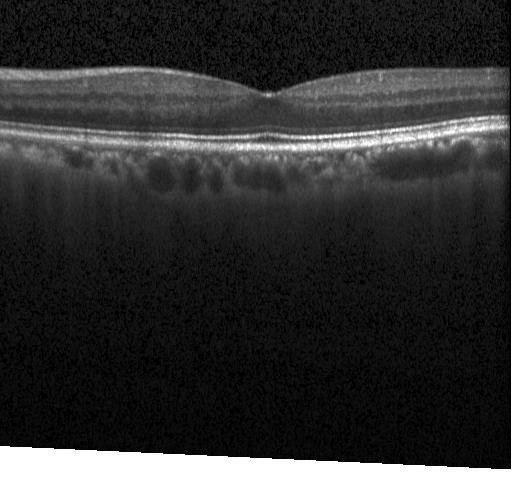
OCT line scan
Assessment: no evidence of choroidal neovascularization, diabetic macular edema, or drusen.